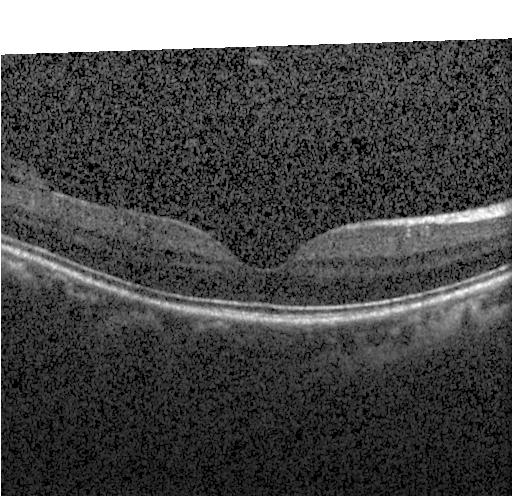 Finding: neither CNV, DME, nor drusen.